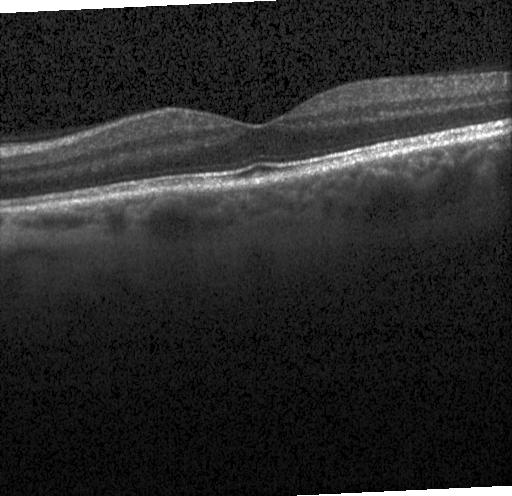
Spectral-domain optical coherence tomography. Macular scan. Retinal OCT B-scan. Acquired on a Heidelberg Spectralis
Diagnosis: neither CNV, DME, nor drusen.